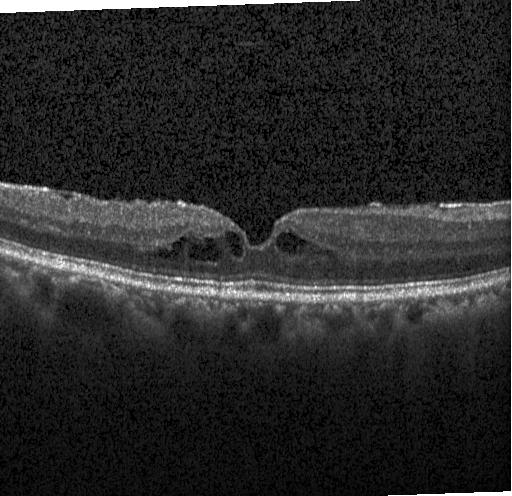 OCT B-scan · through the macula
Diabetic macular edema (DME).